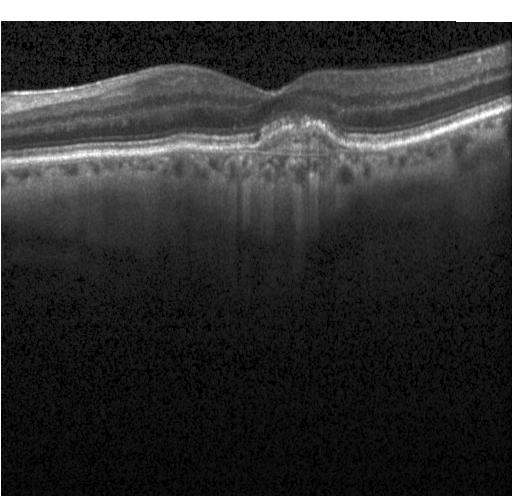
Finding: a choroidal neovascular membrane.